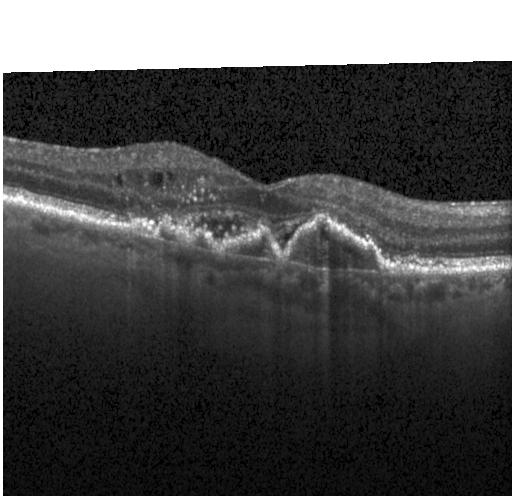 This B-scan demonstrates a choroidal neovascular membrane.